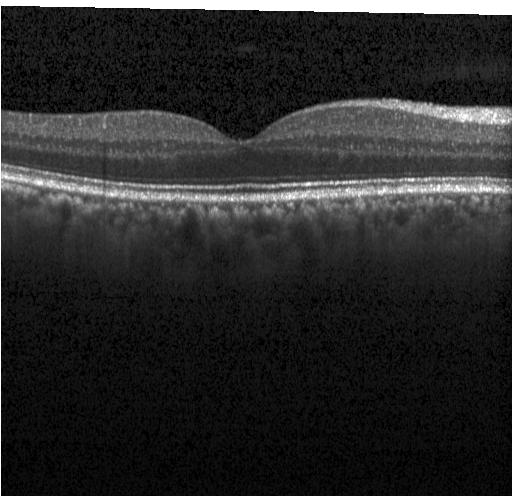

Dx: neither CNV, DME, nor drusen.